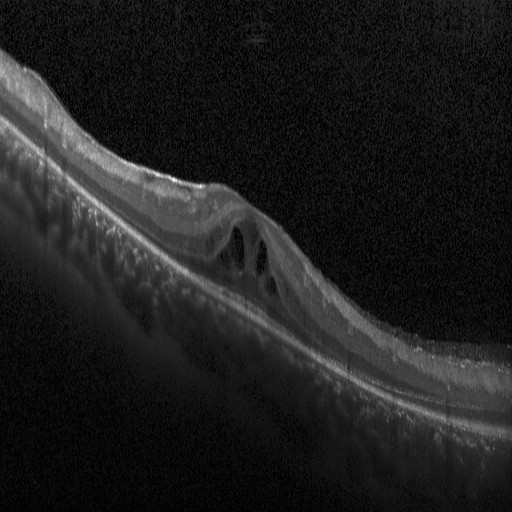
Through the macula. Retinal OCT cross-section. Spectral-domain optical coherence tomography. Heidelberg Spectralis OCT system. Finding: diabetic macular edema (DME).